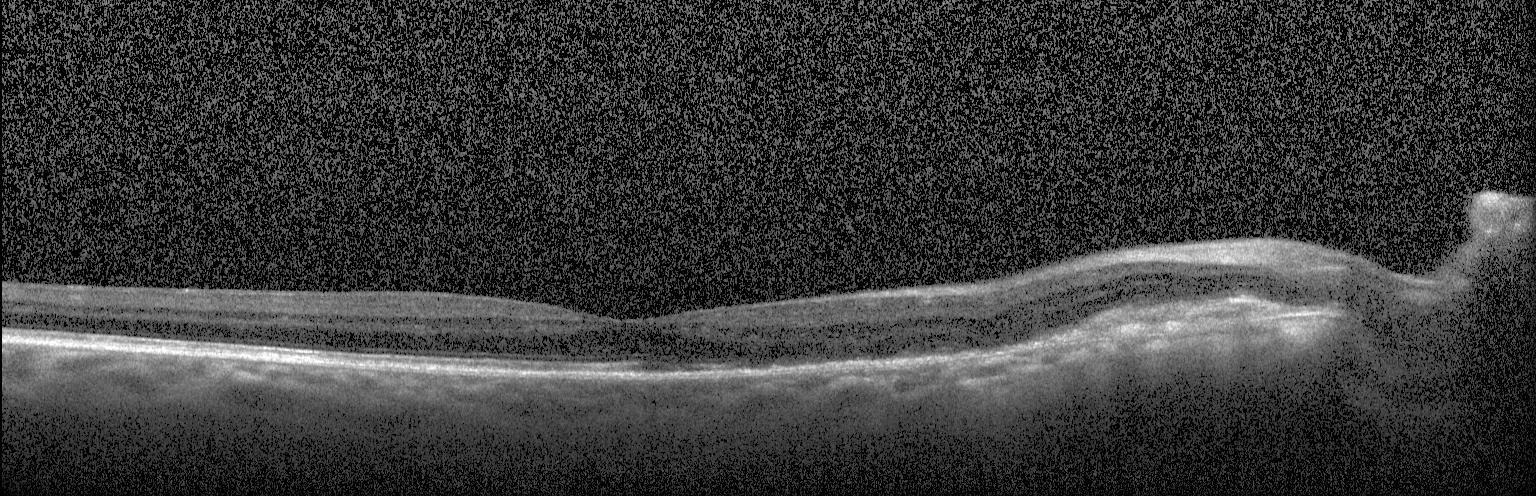

Diagnosis: choroidal neovascularization (CNV).